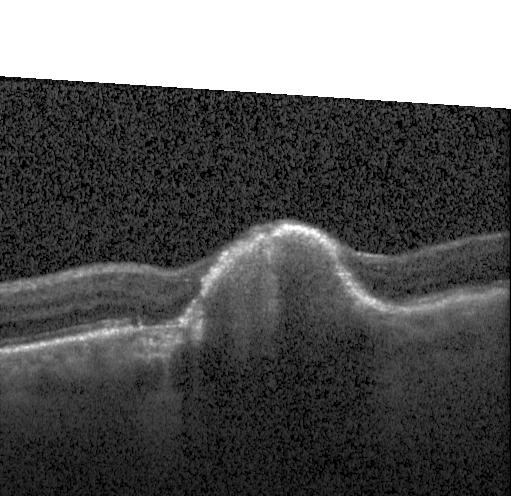 Retinal OCT B-scan. OCT finding: a choroidal neovascular membrane.